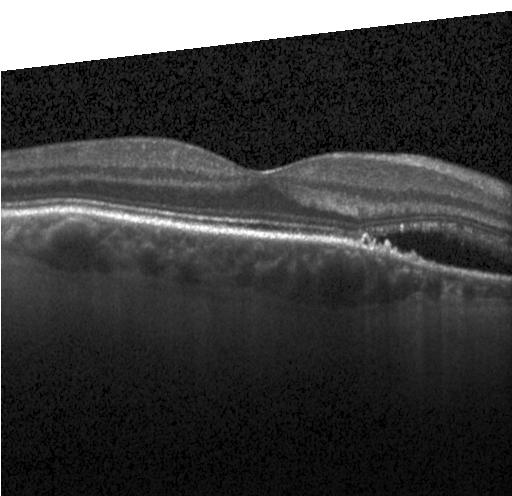
Spectral-domain OCT B-scan: choroidal neovascularization.